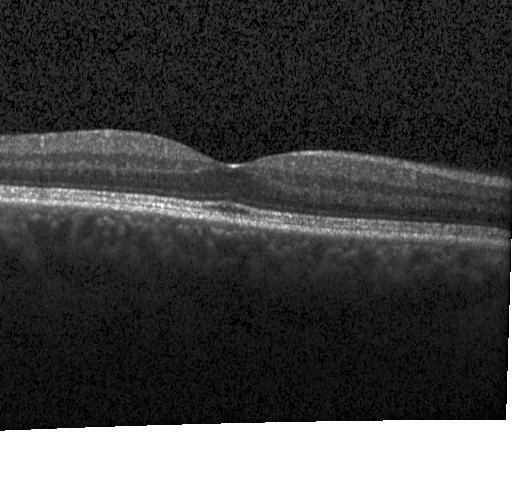

Spectral-domain OCT B-scan: neither choroidal neovascularization, diabetic macular edema, nor drusen.